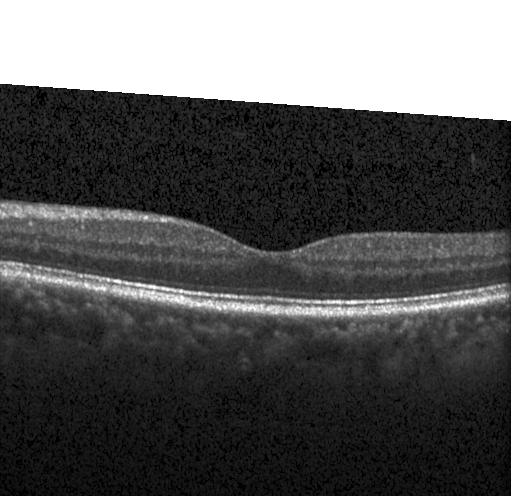 Optical coherence tomography scan — Diagnosis: no evidence of CNV, DME, or drusen.